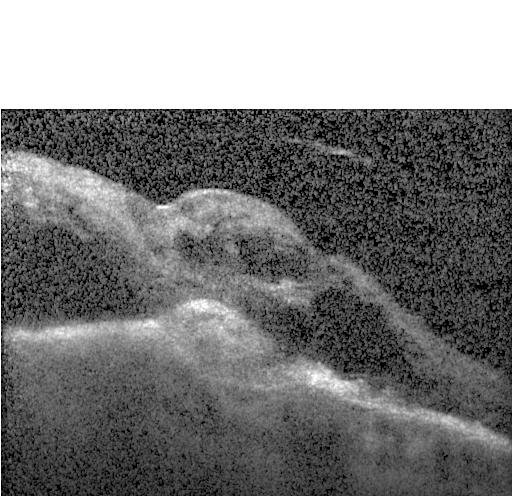

Dx: a choroidal neovascular membrane.